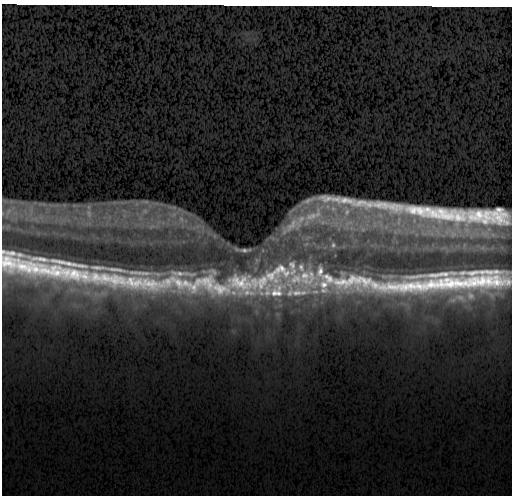
Finding: choroidal neovascularization.